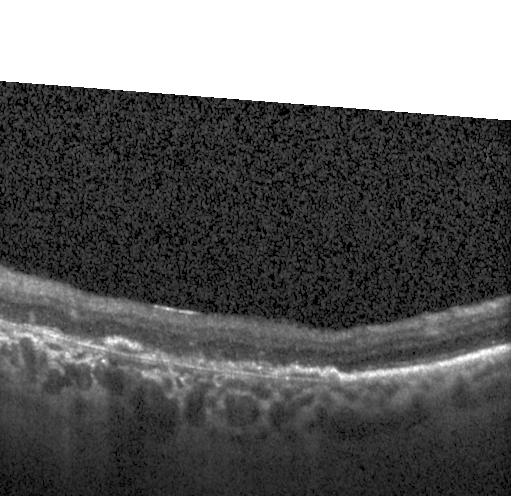 Retinal OCT cross-section
Assessment: a choroidal neovascular membrane.